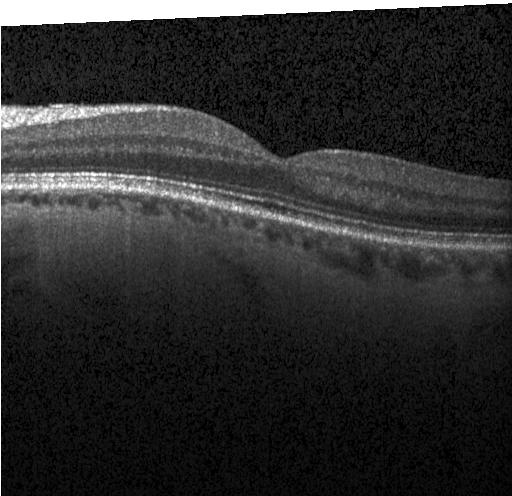 Spectral-domain optical coherence tomography · macular scan · OCT B-scan. Finding: neither choroidal neovascularization, diabetic macular edema, nor drusen.